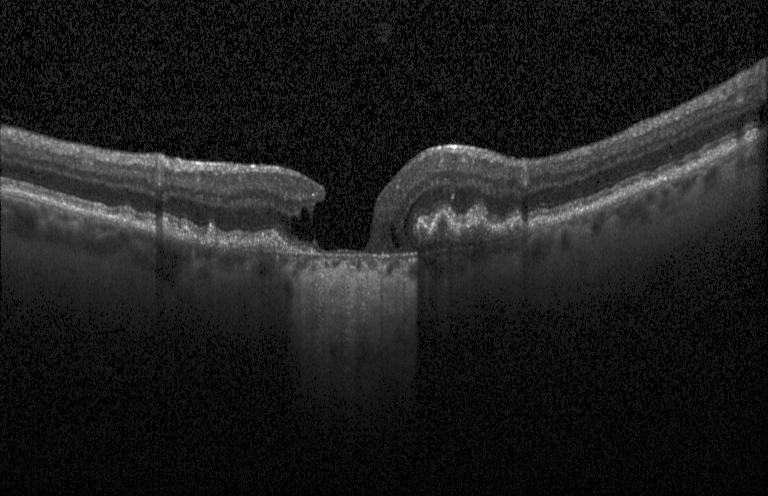

Diagnosis: CNV.